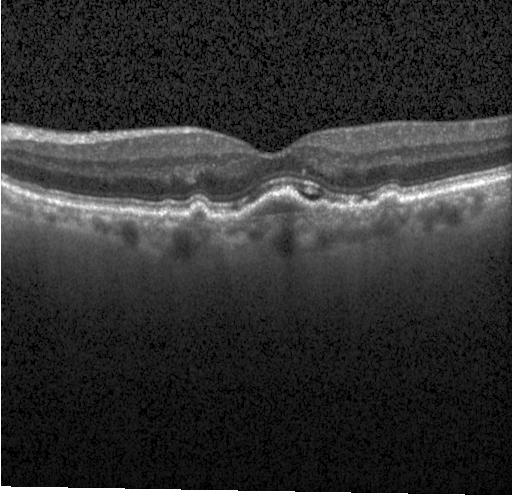
Impression: CNV.